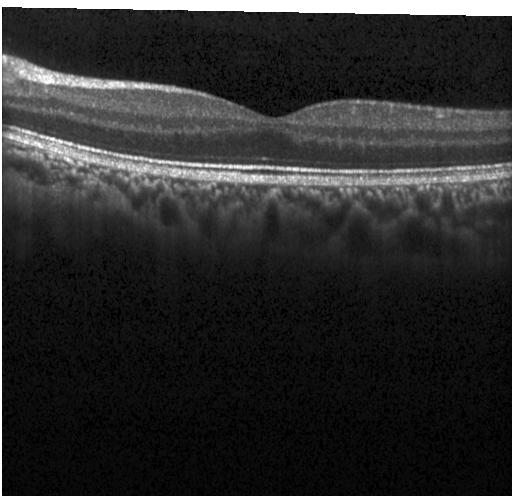 OCT finding: no choroidal neovascularization, no diabetic macular edema, and no drusen.